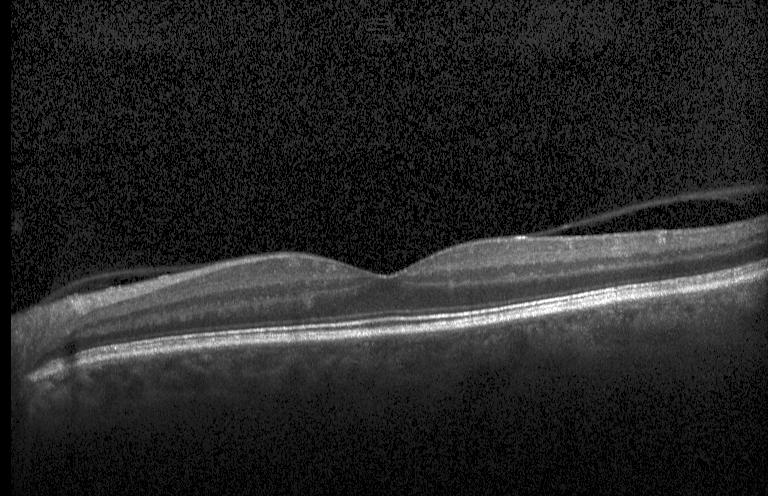

Retinal OCT cross-section. Diagnosis: no CNV, DME, or drusen.